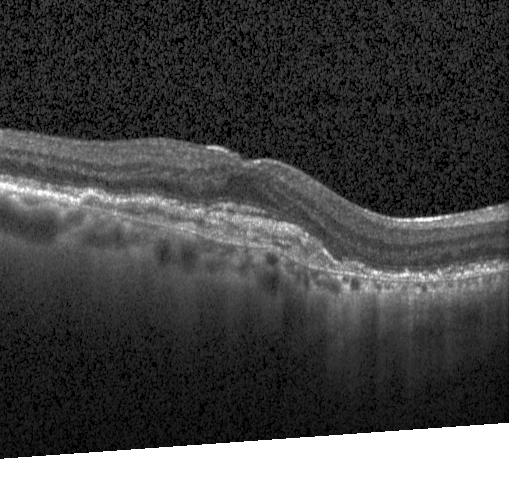
Assessment: CNV.